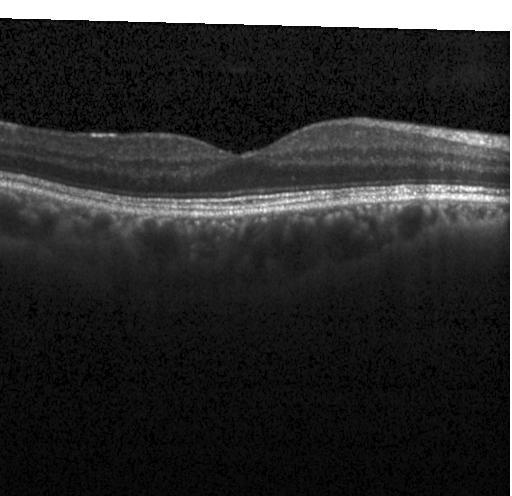 Instrument: Heidelberg Spectralis. SD-OCT. OCT line scan — Finding: no choroidal neovascularization, diabetic macular edema, or drusen.